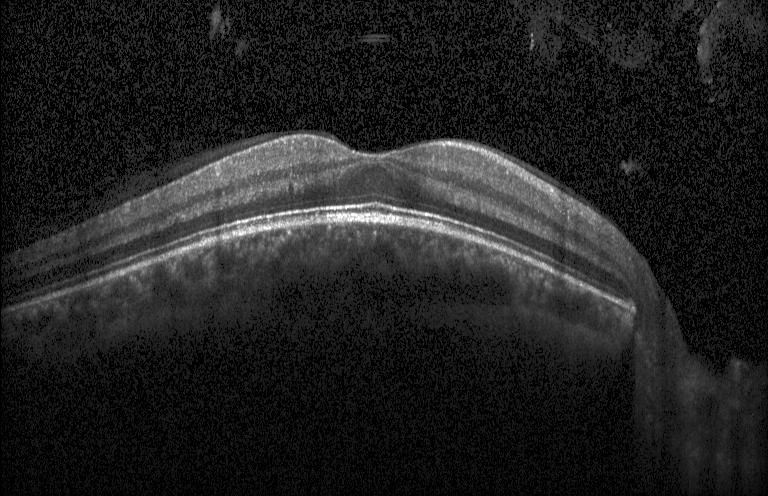

OCT scan showing no choroidal neovascularization, no diabetic macular edema, and no drusen.